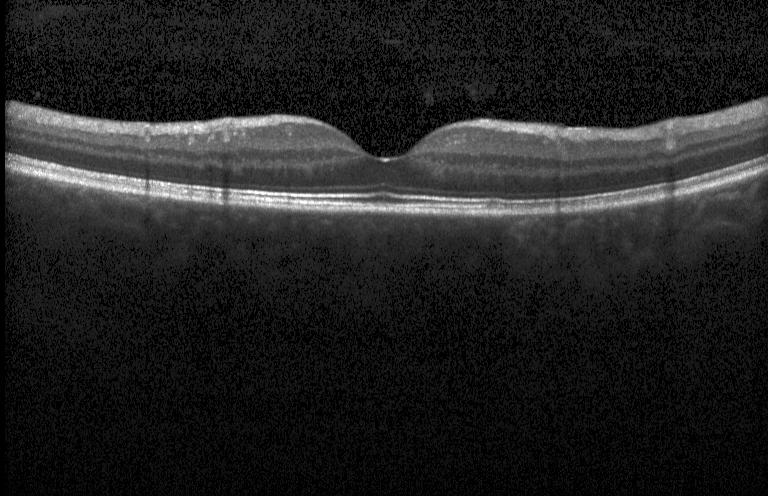
Retinal OCT B-scan, acquired on a Heidelberg Spectralis, fovea-centered, SD-OCT — No choroidal neovascularization, diabetic macular edema, or drusen.